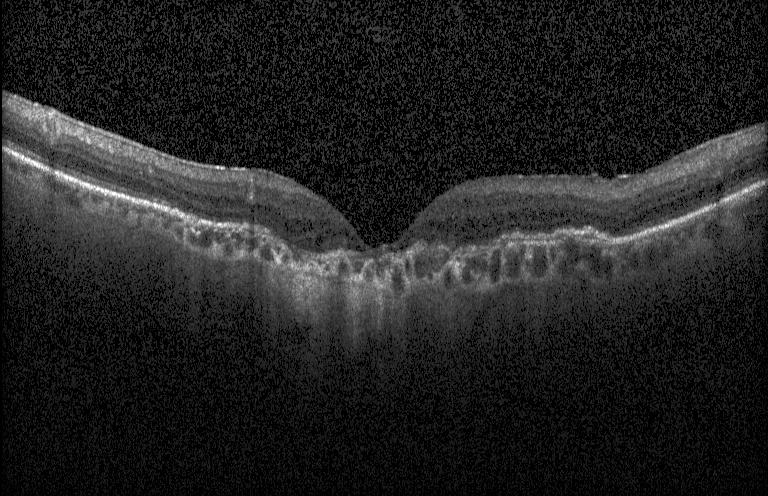
Spectral-domain OCT B-scan: a choroidal neovascular membrane.